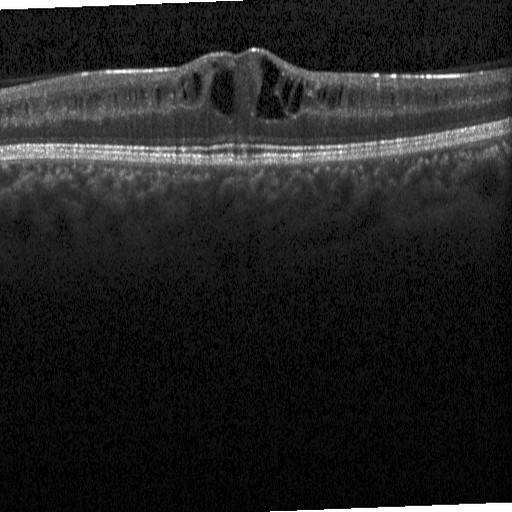

Macular OCT: diabetic macular edema (DME).